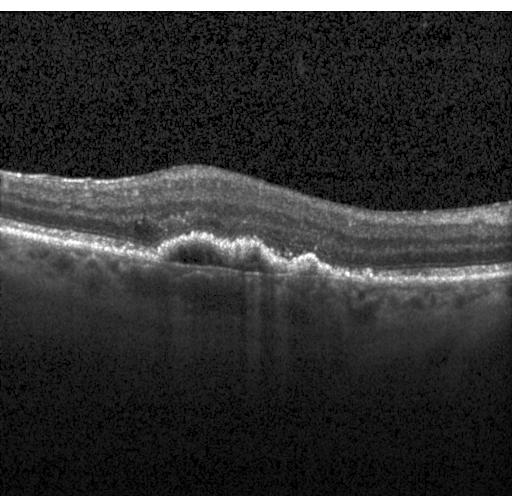

Centered on the fovea; optical coherence tomography B-scan; spectral-domain optical coherence tomography
Macular OCT: choroidal neovascularization.